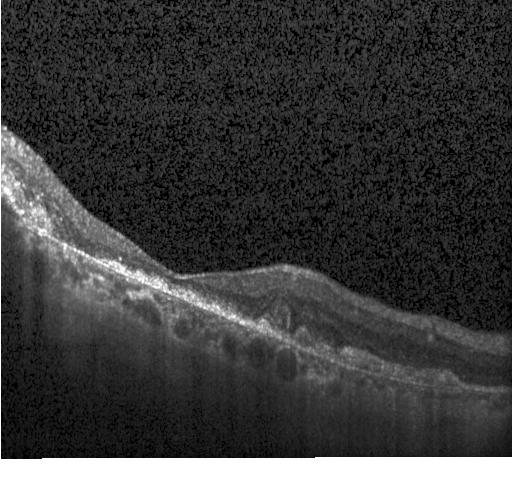 Optical coherence tomography scan, spectral-domain optical coherence tomography
The scan shows a choroidal neovascular membrane.